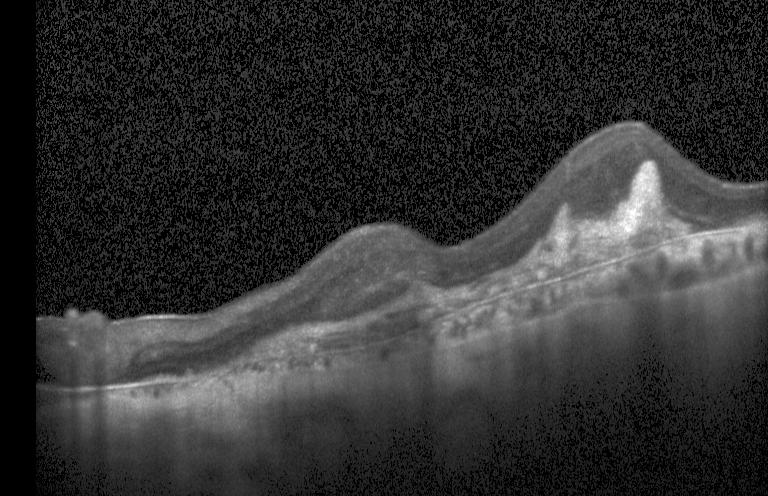
Dx: a choroidal neovascular membrane.